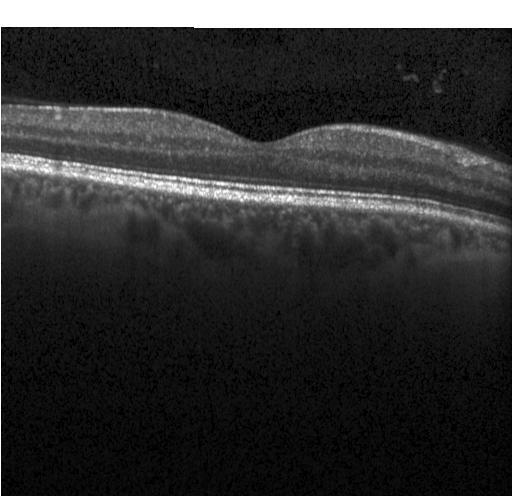 Optical coherence tomography B-scan. Spectral-domain optical coherence tomography. Instrument: Heidelberg Spectralis
Diagnosis: no CNV, no DME, and no drusen.